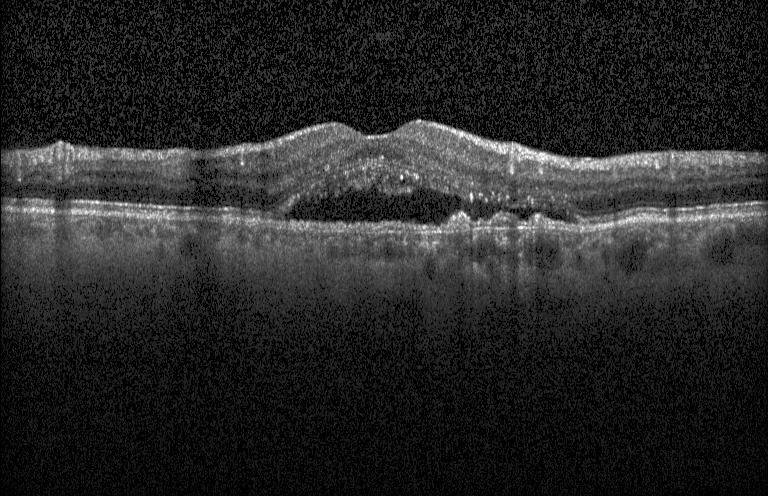
Optical coherence tomography B-scan
The scan shows a choroidal neovascular membrane.